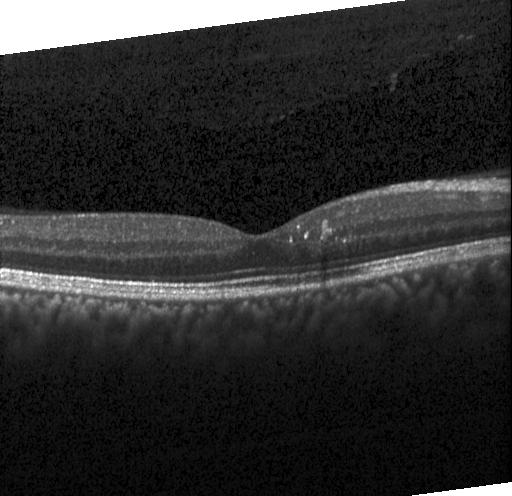 Diagnosis: no choroidal neovascularization, diabetic macular edema, or drusen.